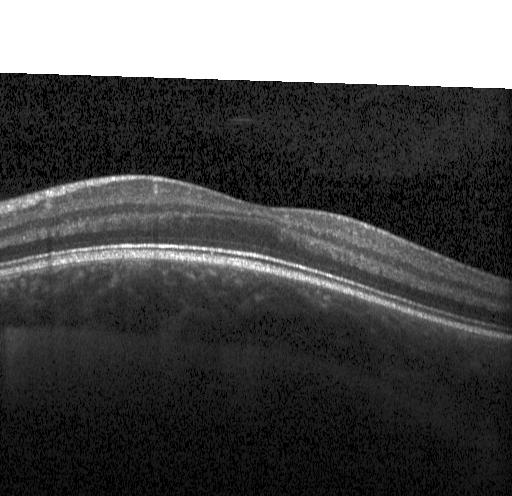

Optical coherence tomography scan · horizontal scan through the fovea
Neither choroidal neovascularization, diabetic macular edema, nor drusen.